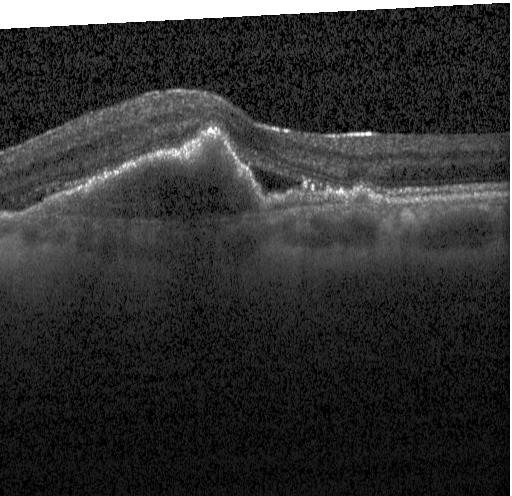
Retinal OCT B-scan · fovea-centered. Macular OCT: a choroidal neovascular membrane.